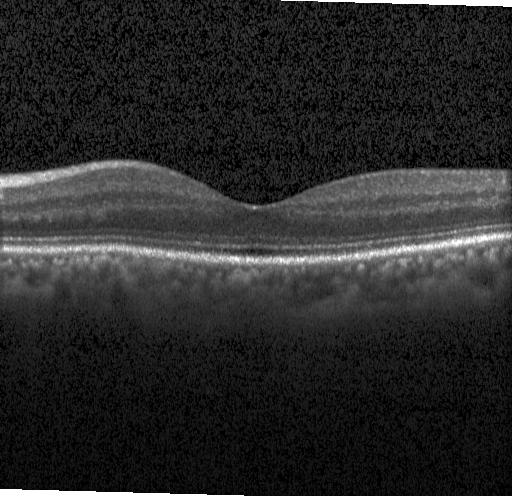

Dx: neither CNV, DME, nor drusen.